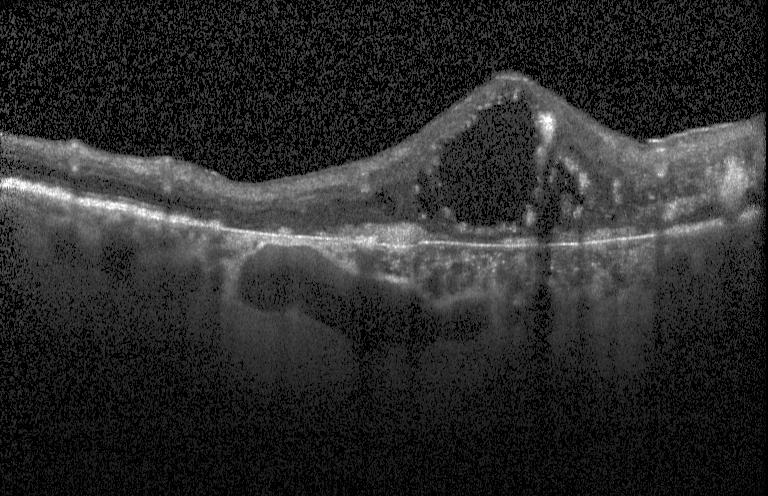 SD-OCT; optical coherence tomography scan — Finding: a choroidal neovascular membrane.